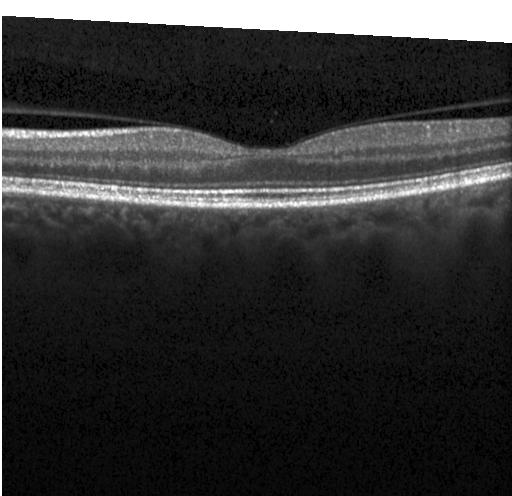
Spectral-domain OCT B-scan: no choroidal neovascularization, no diabetic macular edema, and no drusen.